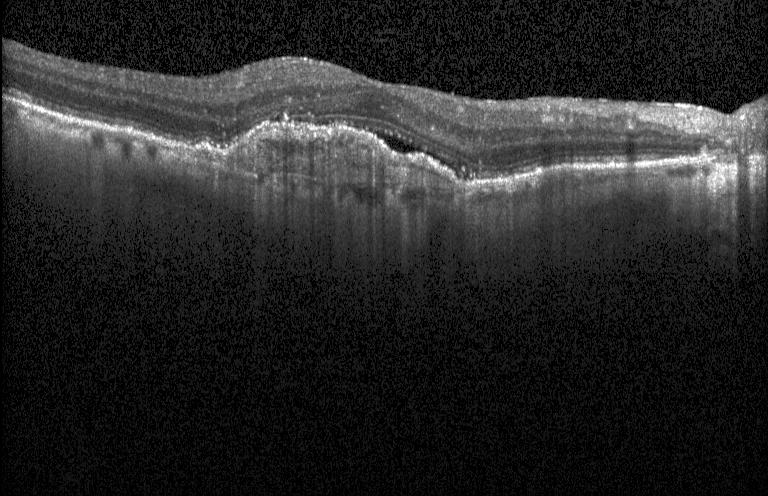 Heidelberg Spectralis OCT system · SD-OCT · optical coherence tomography scan. Dx: a choroidal neovascular membrane.